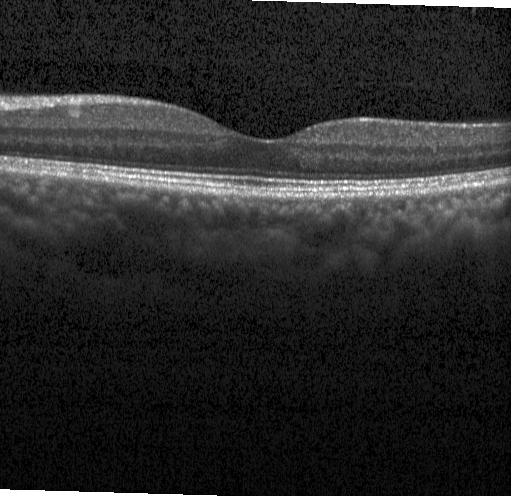

Acquired on a Heidelberg Spectralis, optical coherence tomography scan, through the macula — No evidence of CNV, DME, or drusen.